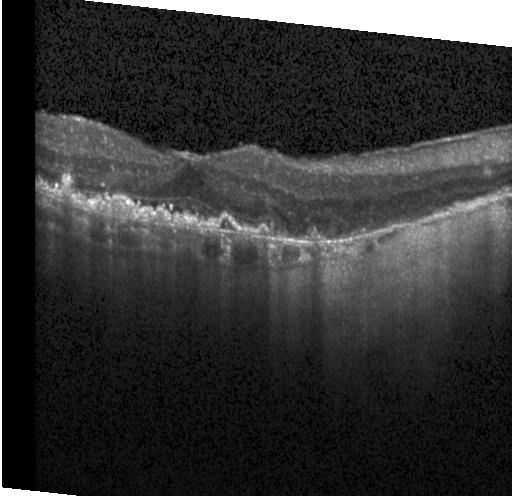

Centered on the fovea · OCT B-scan · acquired on a Heidelberg Spectralis
Dx: choroidal neovascularization.